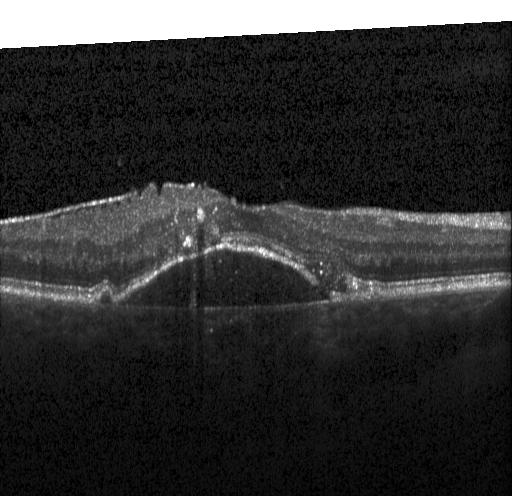

OCT finding: a choroidal neovascular membrane.